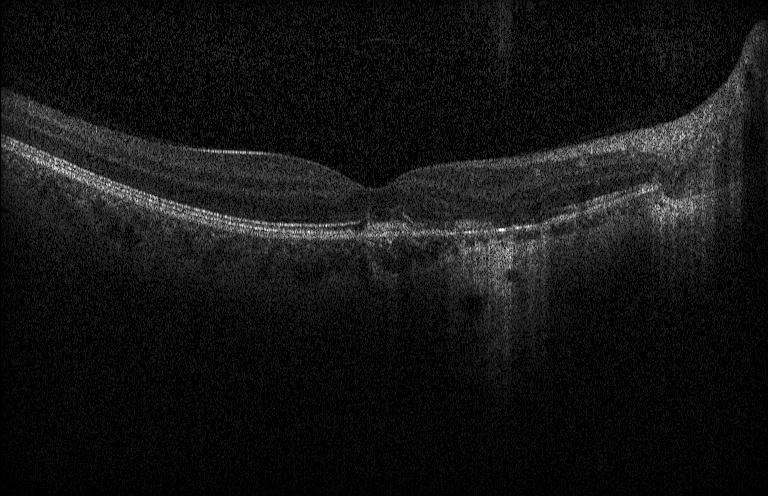 OCT B-scan showing choroidal neovascularization.